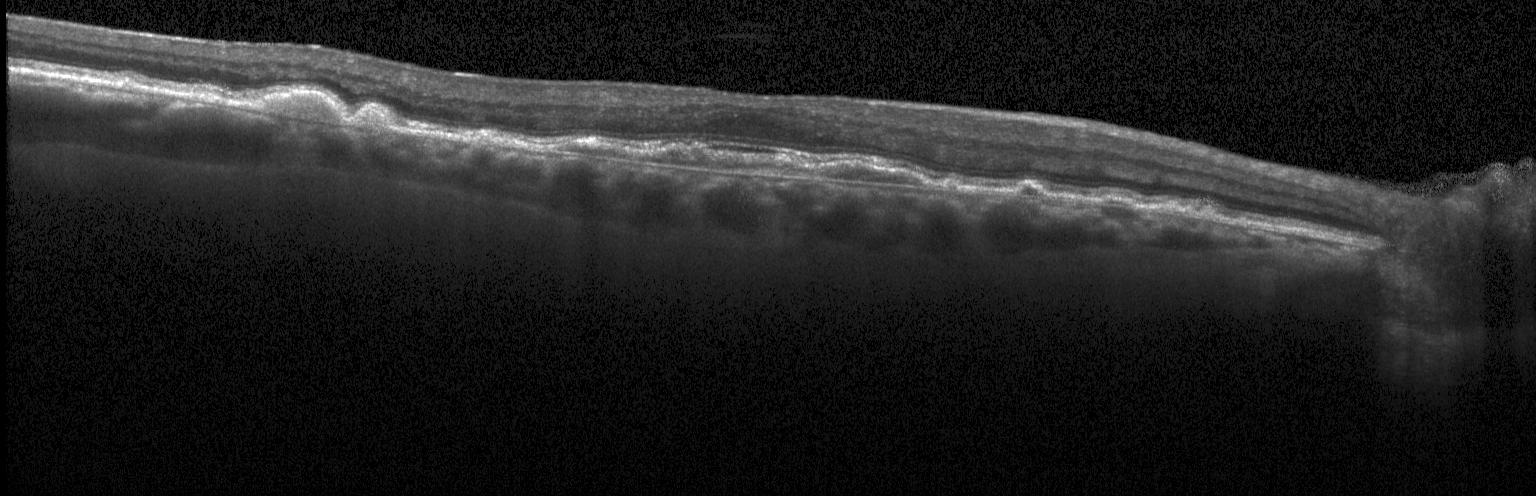

Heidelberg Spectralis OCT system. Optical coherence tomography B-scan. Spectral-domain OCT.
A choroidal neovascular membrane.